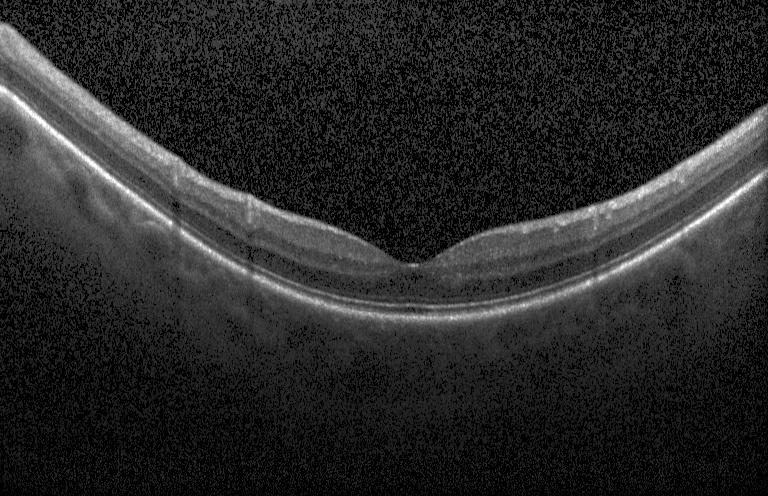
Neither choroidal neovascularization, diabetic macular edema, nor drusen.